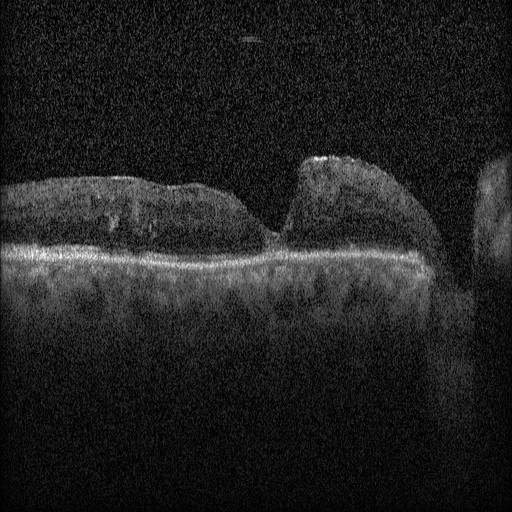 Impression: diabetic macular edema (DME).